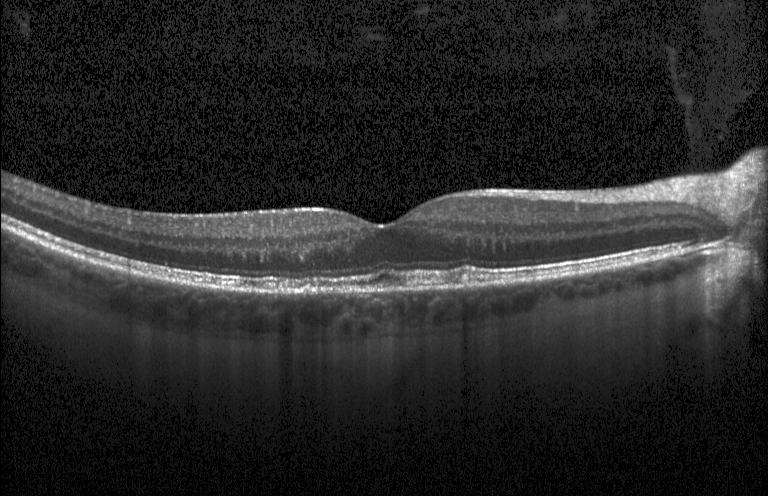 Retinal OCT B-scan; acquired on a Heidelberg Spectralis.
Finding: sub-RPE drusenoid deposits.